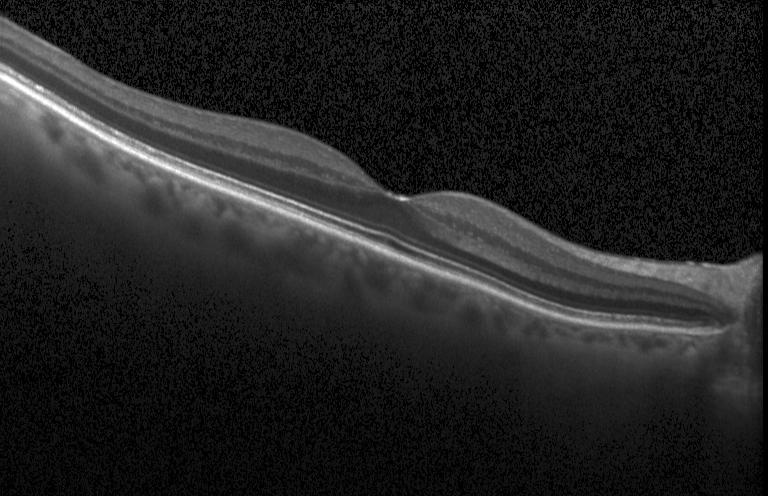 Optical coherence tomography scan. Finding: neither CNV, DME, nor drusen.